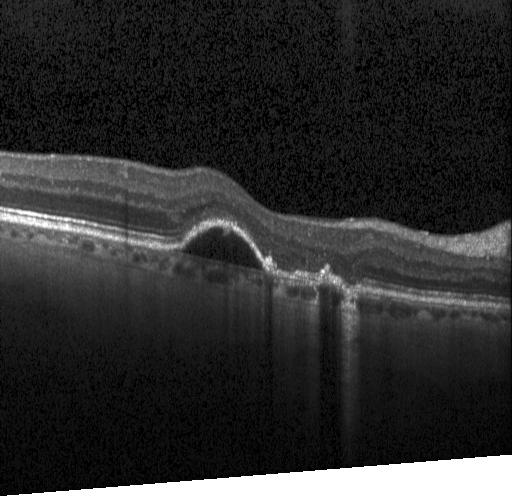

Instrument: Heidelberg Spectralis, OCT line scan, SD-OCT, horizontal scan through the fovea — Impression: CNV.